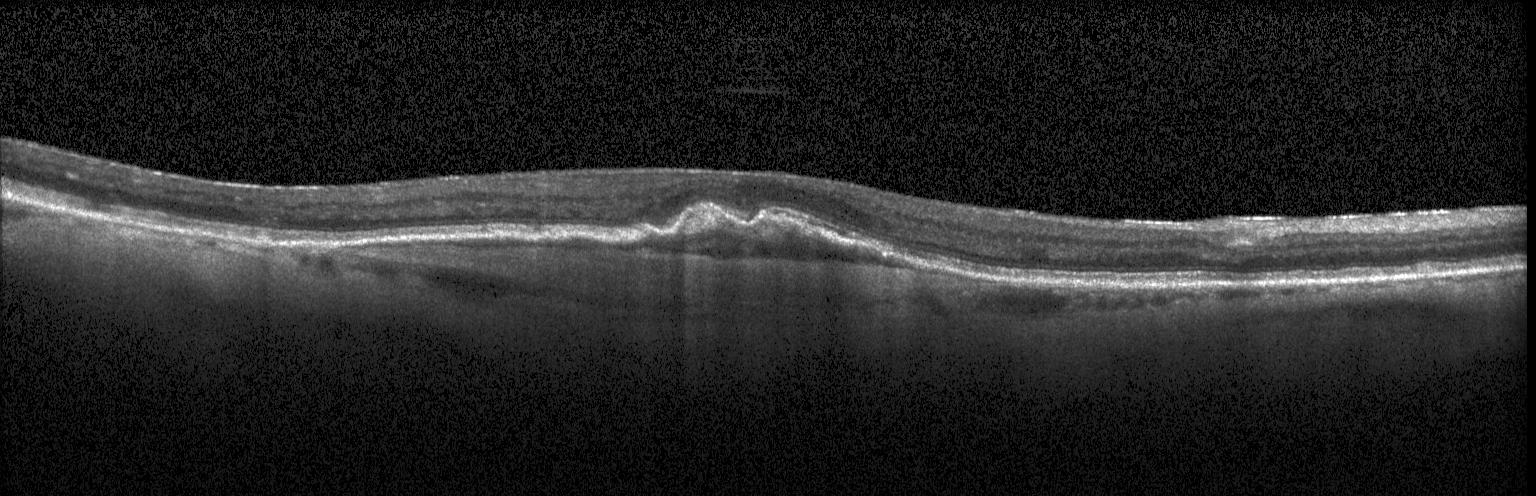

OCT finding: choroidal neovascularization.